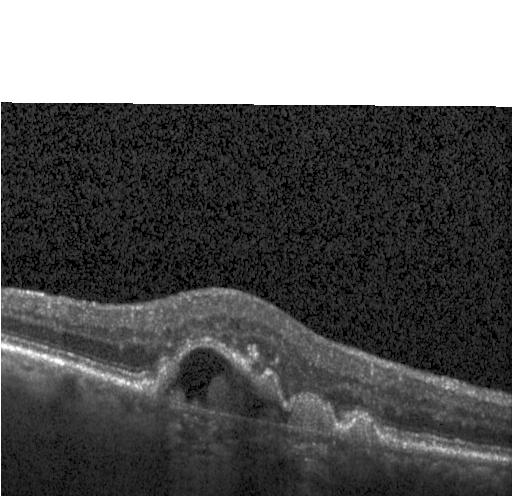

Retinal OCT B-scan. Macular scan
The scan shows a choroidal neovascular membrane.